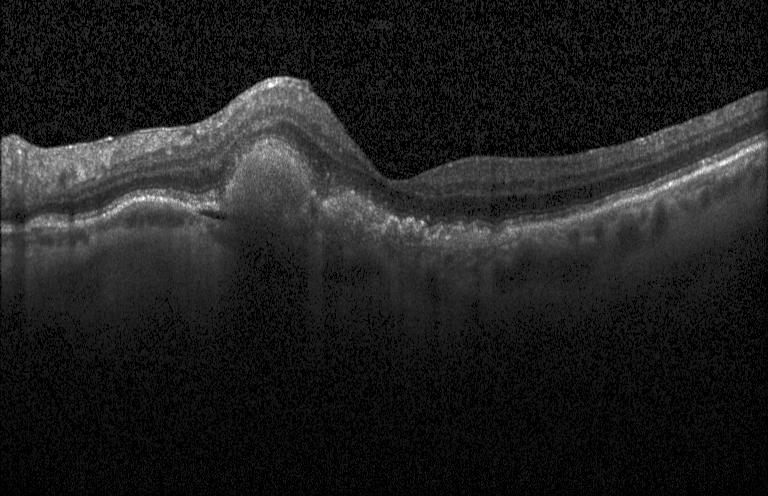
Macular OCT: choroidal neovascularization.